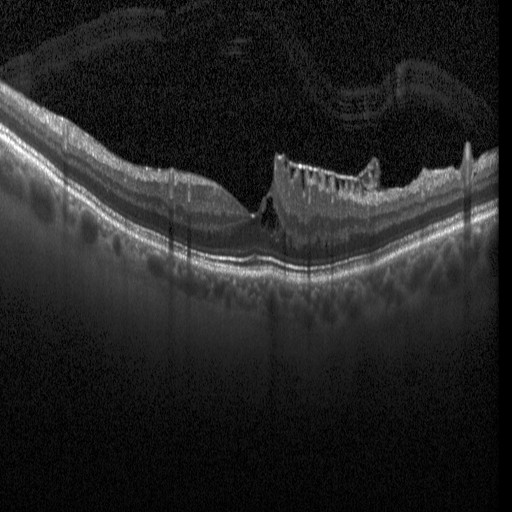

Retinal OCT cross-section; spectral-domain OCT; acquired on a Heidelberg Spectralis; centered on the fovea
Diabetic macular edema (DME).